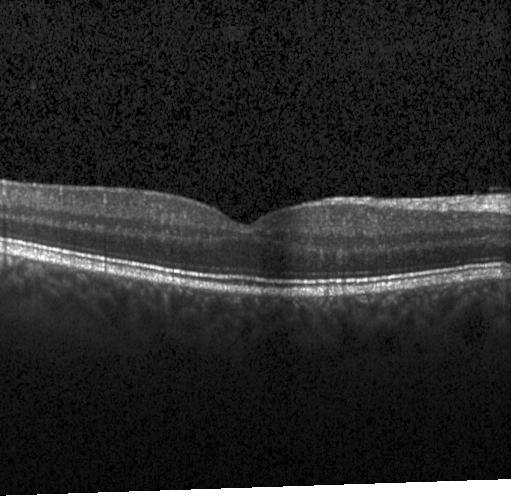
Horizontal scan through the fovea, optical coherence tomography scan, acquired on a Heidelberg Spectralis — Impression: no choroidal neovascularization, diabetic macular edema, or drusen.